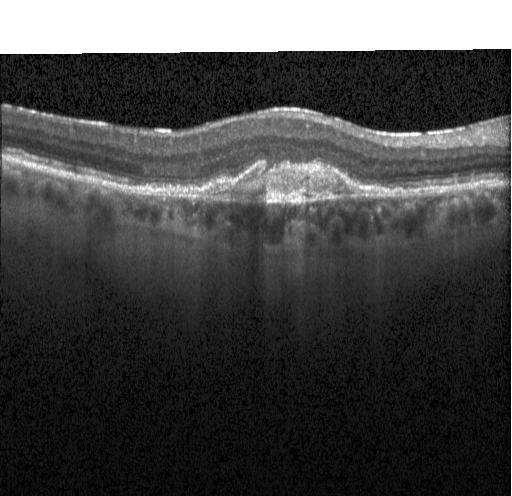
Acquired on a Heidelberg Spectralis, spectral-domain optical coherence tomography, OCT line scan — Finding: a choroidal neovascular membrane.